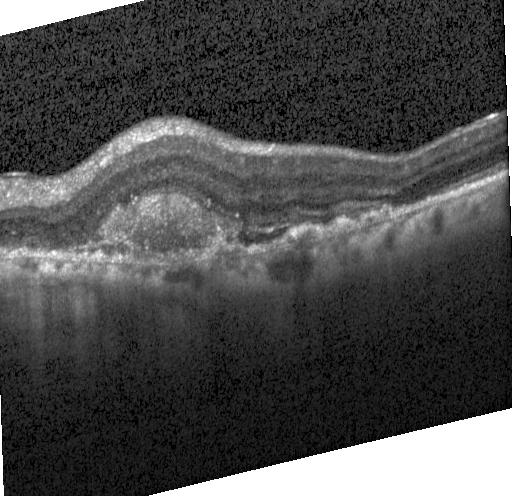 Retinal OCT cross-section. Spectral-domain optical coherence tomography. Heidelberg Spectralis OCT system — This B-scan demonstrates a choroidal neovascular membrane.